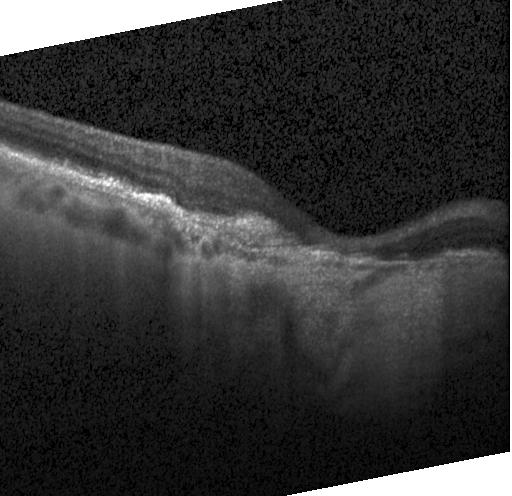 Spectral-domain OCT, centered on the fovea, retinal OCT cross-section
Impression: choroidal neovascularization.